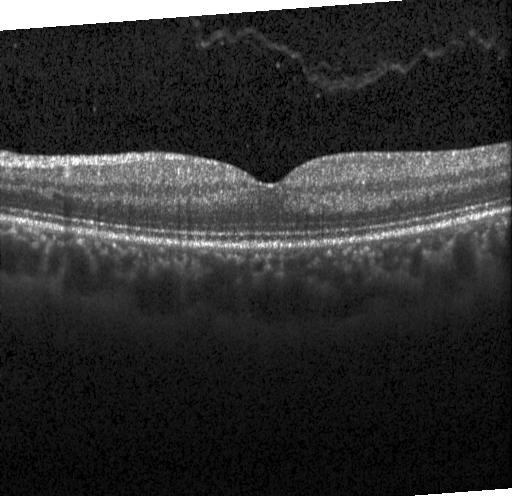
Acquired on a Heidelberg Spectralis · SD-OCT · horizontal scan through the fovea · optical coherence tomography scan — Finding: no evidence of choroidal neovascularization, diabetic macular edema, or drusen.